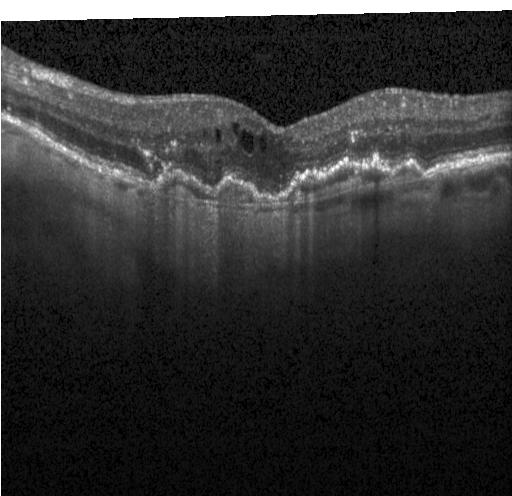

Finding: a choroidal neovascular membrane.